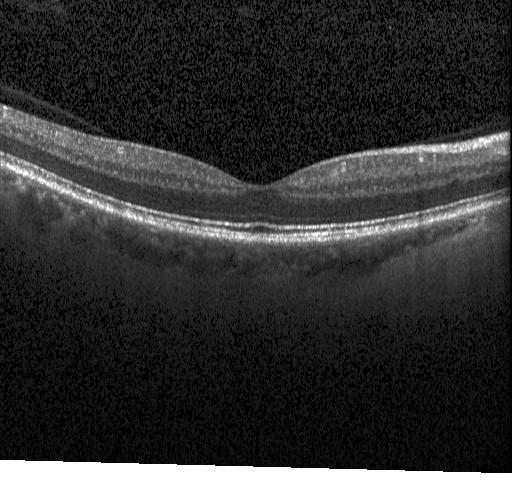
Optical coherence tomography scan. SD-OCT. Impression: no choroidal neovascularization, no diabetic macular edema, and no drusen.